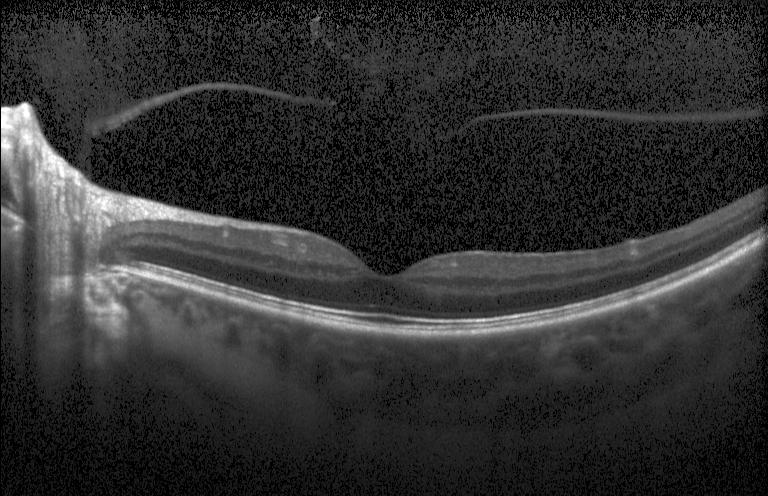 Horizontal scan through the fovea, acquired on a Heidelberg Spectralis, optical coherence tomography scan, SD-OCT
Assessment: no evidence of choroidal neovascularization, diabetic macular edema, or drusen.